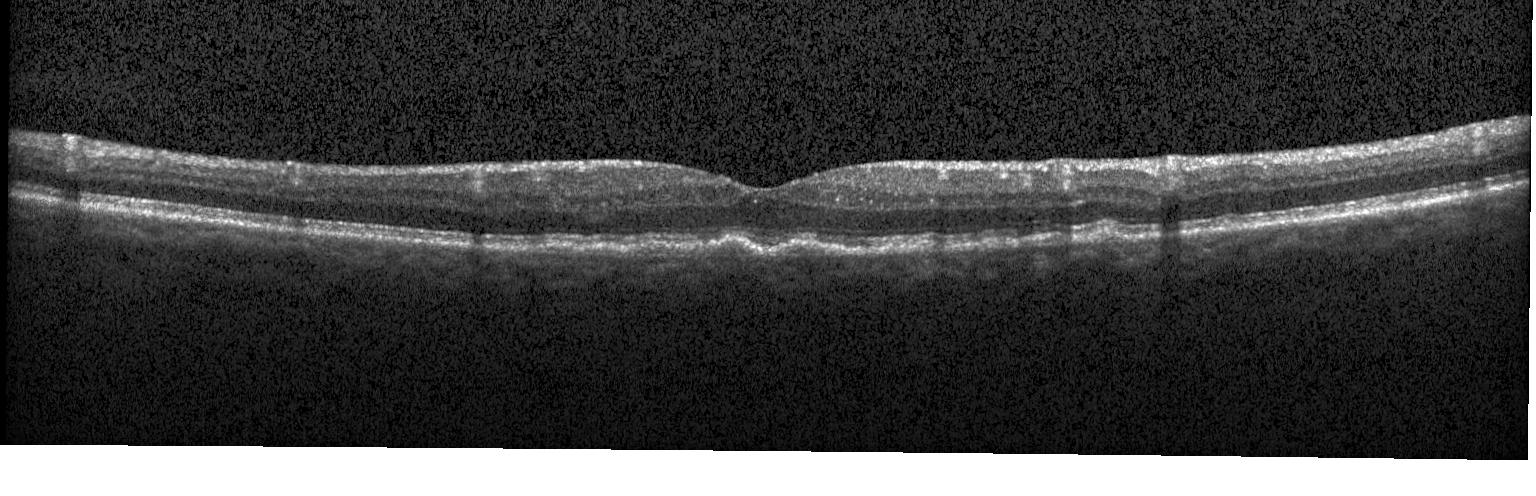
Heidelberg Spectralis OCT system · through the macula · OCT B-scan
Macular OCT: sub-RPE drusenoid deposits.